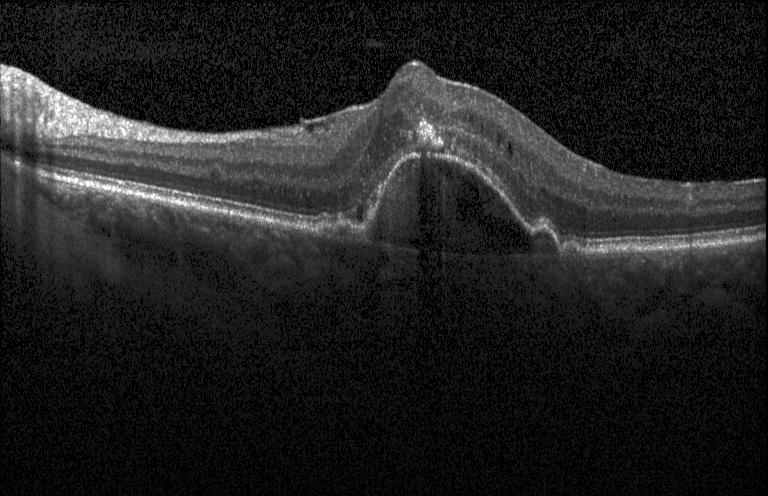 Optical coherence tomography B-scan.
Impression: a choroidal neovascular membrane.